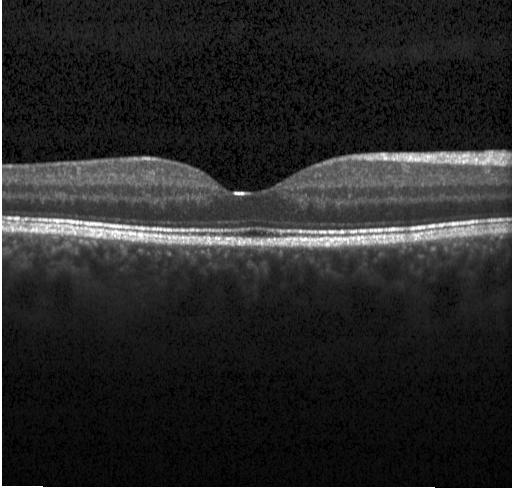
Retinal OCT B-scan. Heidelberg Spectralis. Centered on the fovea.
Dx: neither choroidal neovascularization, diabetic macular edema, nor drusen.